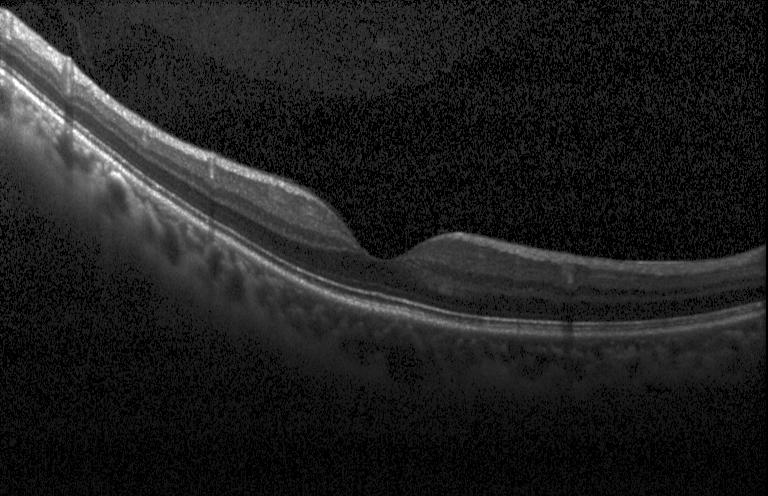 OCT line scan — This B-scan demonstrates neither choroidal neovascularization, diabetic macular edema, nor drusen.